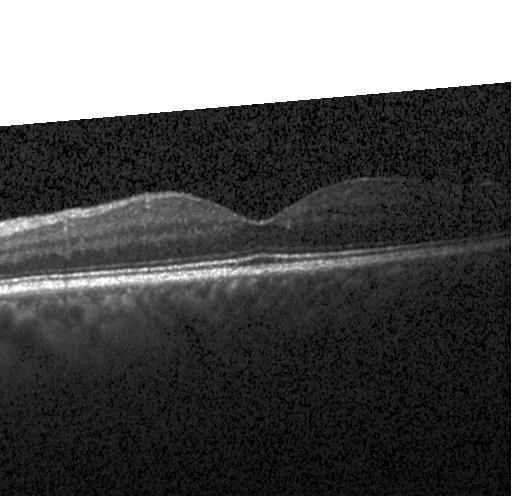

Neither choroidal neovascularization, diabetic macular edema, nor drusen.